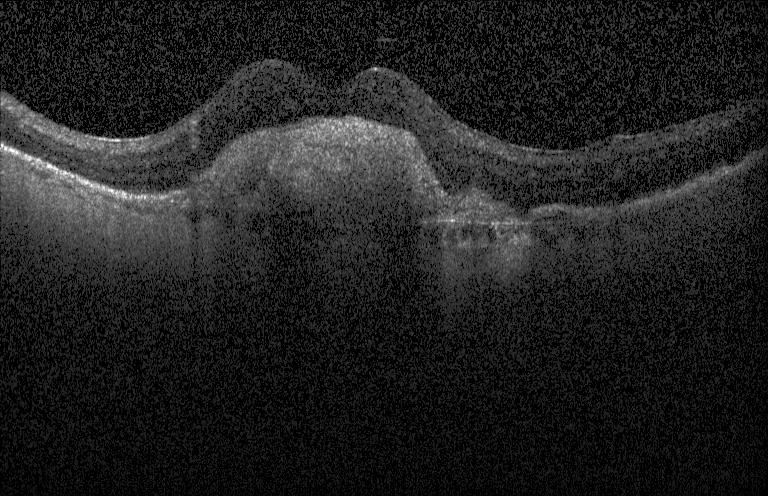

Horizontal scan through the fovea · spectral-domain OCT · OCT line scan
Choroidal neovascularization (CNV).